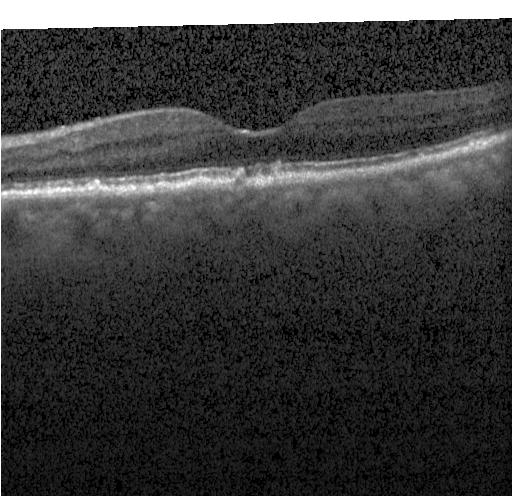

Finding: multiple drusen.